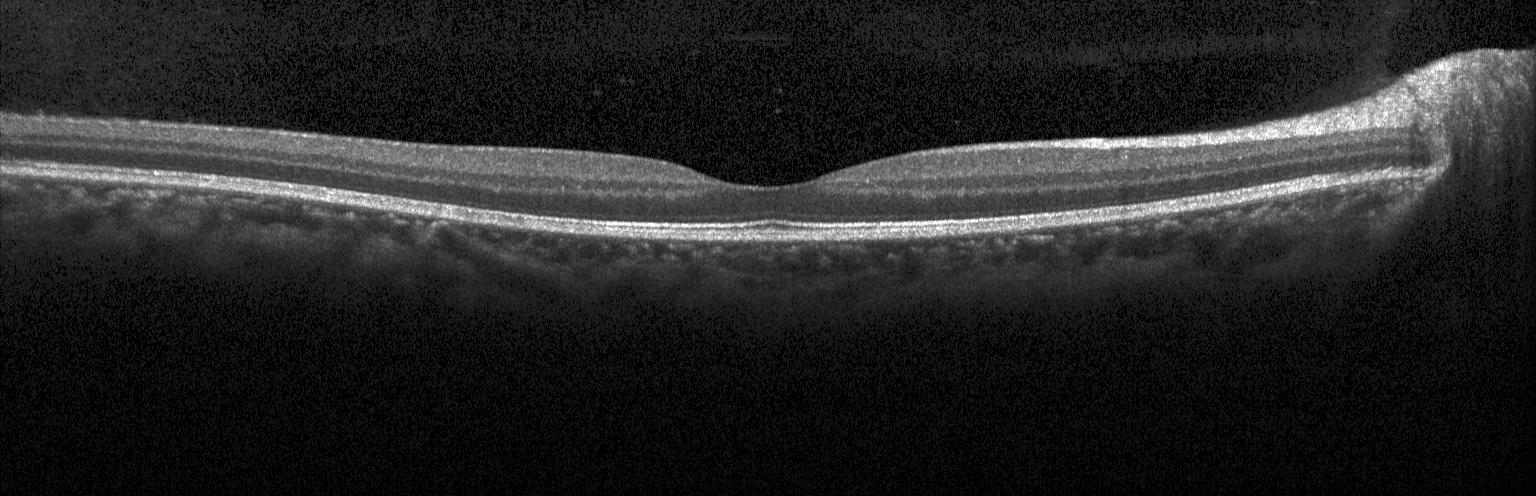 Optical coherence tomography scan; SD-OCT — The scan shows no choroidal neovascularization, no diabetic macular edema, and no drusen.